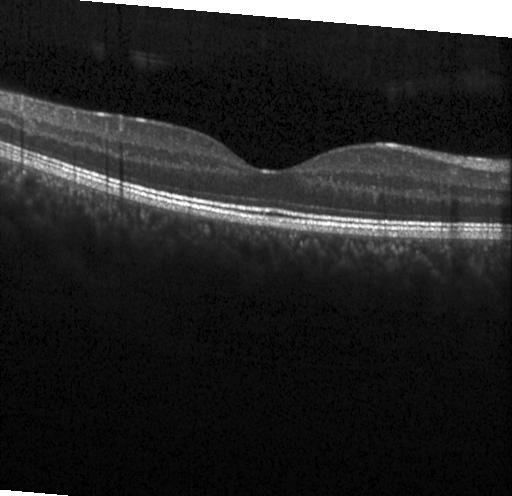 SD-OCT, OCT line scan, macular scan, Heidelberg Spectralis.
Impression: no choroidal neovascularization, no diabetic macular edema, and no drusen.